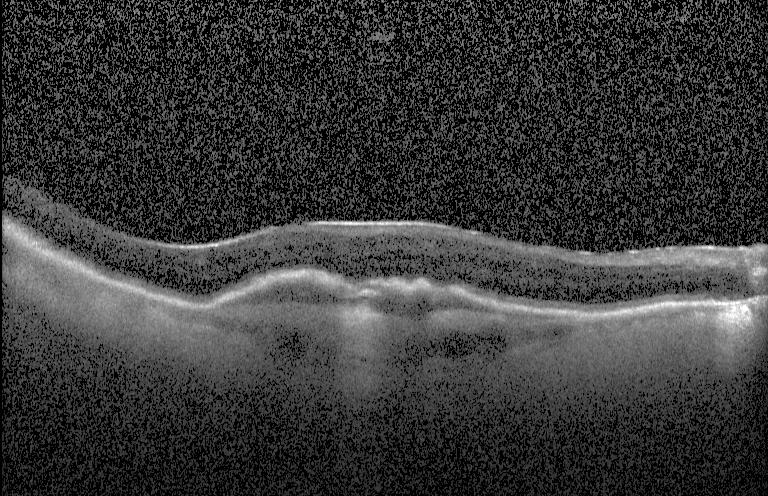
Spectral-domain OCT; acquired on a Heidelberg Spectralis; optical coherence tomography B-scan — This B-scan demonstrates CNV.